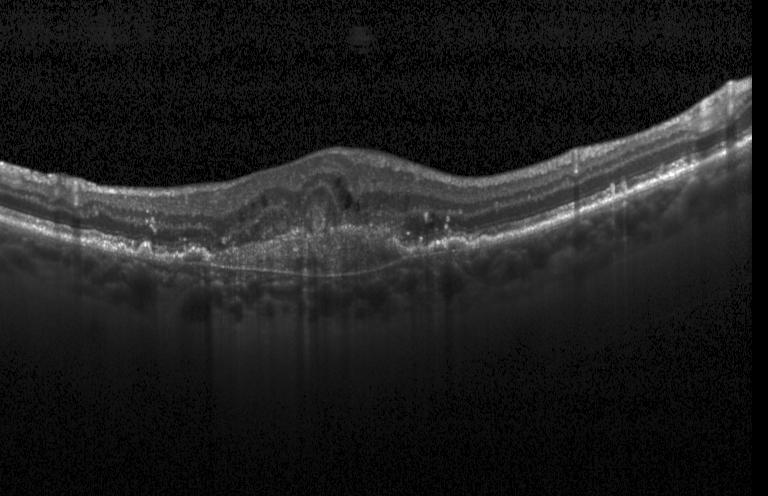

Optical coherence tomography B-scan
Assessment: choroidal neovascularization (CNV).